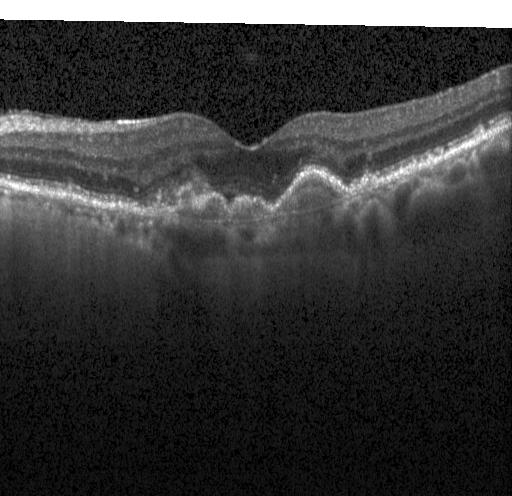 Heidelberg Spectralis OCT system · centered on the fovea · optical coherence tomography scan
A choroidal neovascular membrane.